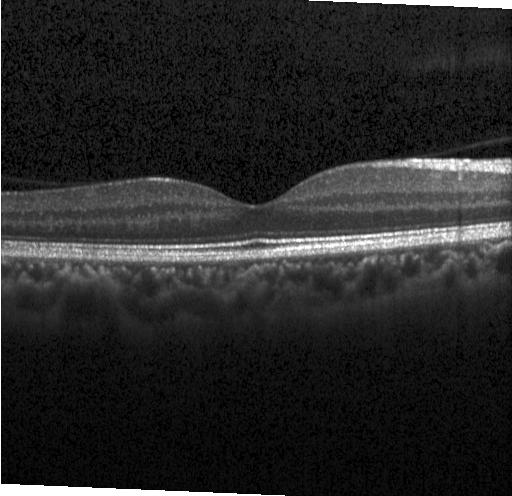

Macular OCT: no evidence of choroidal neovascularization, diabetic macular edema, or drusen.